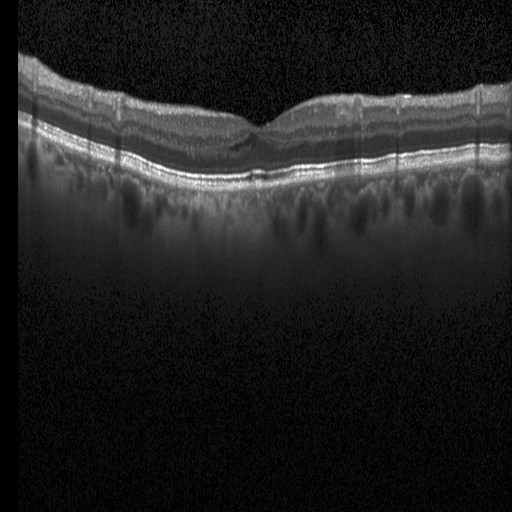
Retinal OCT B-scan, SD-OCT
Diabetic macular edema.